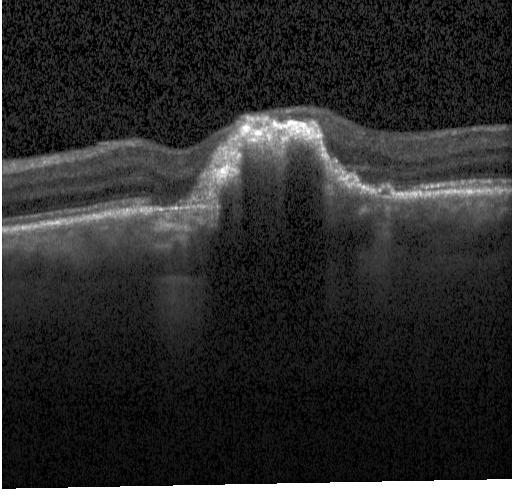 Instrument: Heidelberg Spectralis · retinal OCT cross-section.
Assessment: CNV.